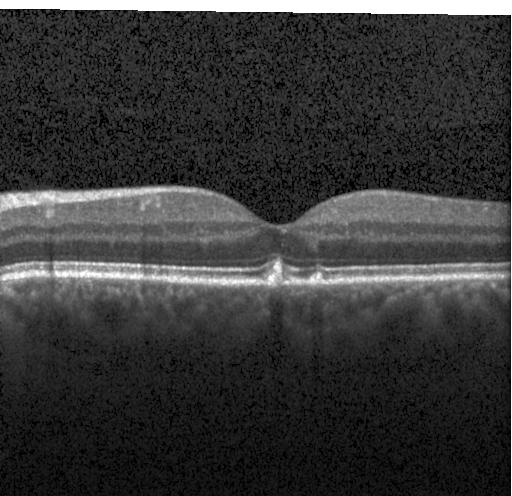

Instrument: Heidelberg Spectralis, retinal OCT B-scan.
Multiple drusen.